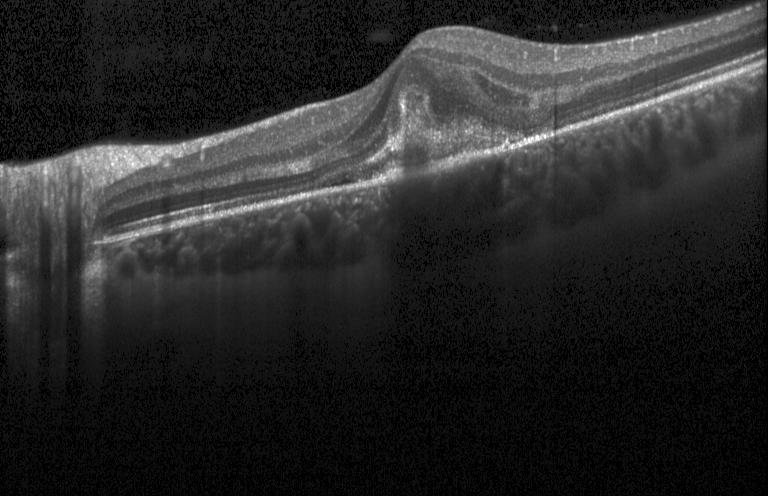 OCT finding: a choroidal neovascular membrane.